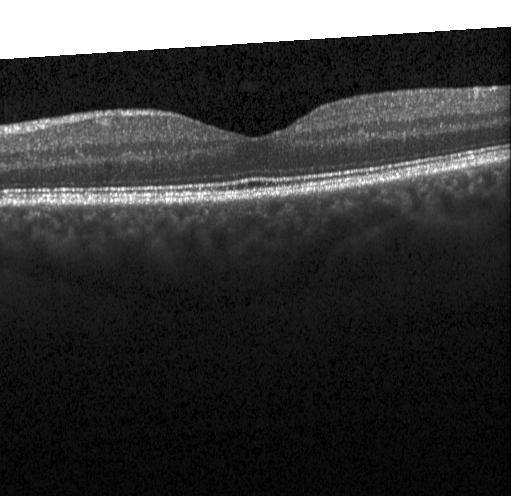

Retinal OCT B-scan. Heidelberg Spectralis OCT system. Through the macula. Spectral-domain OCT — Finding: no CNV, DME, or drusen.